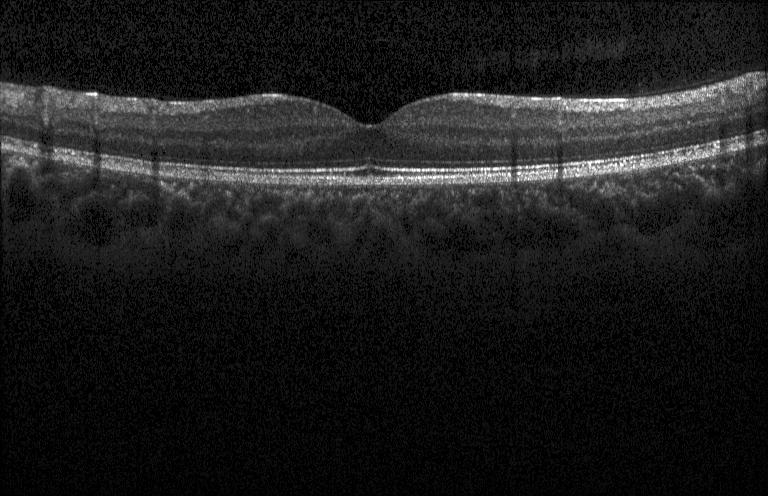
Heidelberg Spectralis · retinal OCT cross-section. This B-scan demonstrates neither choroidal neovascularization, diabetic macular edema, nor drusen.